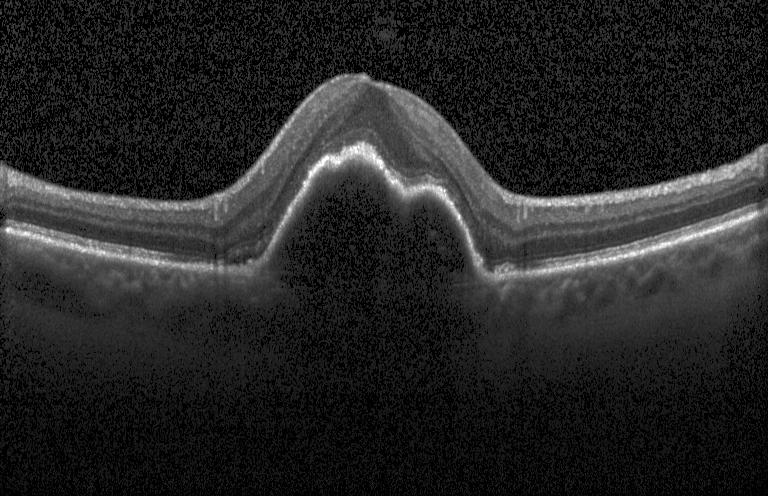 Fovea-centered. Optical coherence tomography scan. Spectral-domain OCT — Finding: a choroidal neovascular membrane.